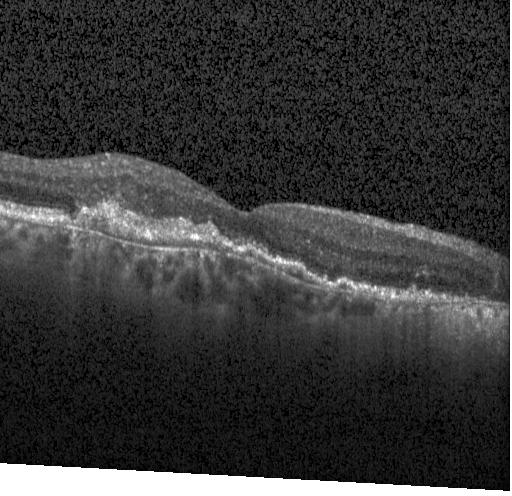
Finding: choroidal neovascularization.